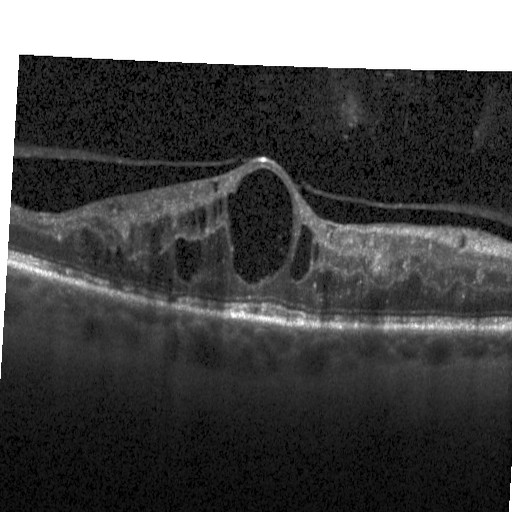
Macular OCT demonstrating diabetic macular edema.